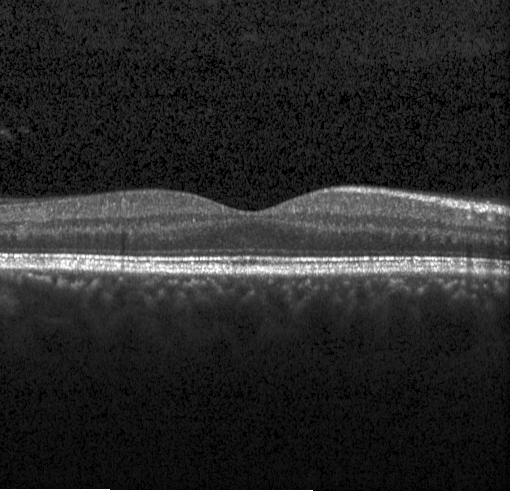
Optical coherence tomography B-scan · spectral-domain OCT
The scan shows neither choroidal neovascularization, diabetic macular edema, nor drusen.